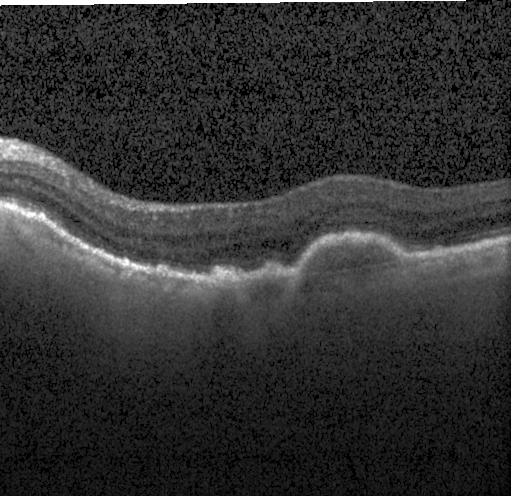

OCT line scan. Spectral-domain OCT. Finding: choroidal neovascularization (CNV).